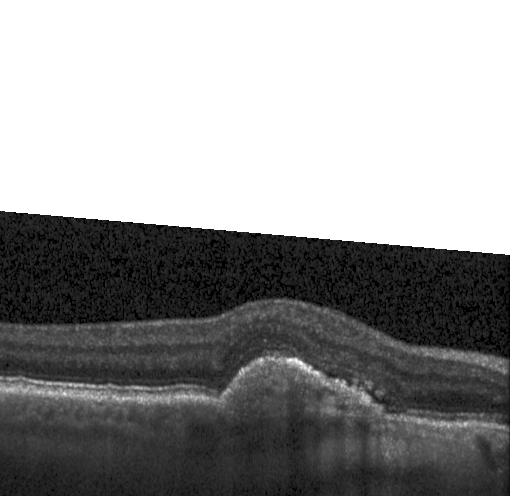
Optical coherence tomography scan. Acquired on a Heidelberg Spectralis. SD-OCT
Dx: CNV.